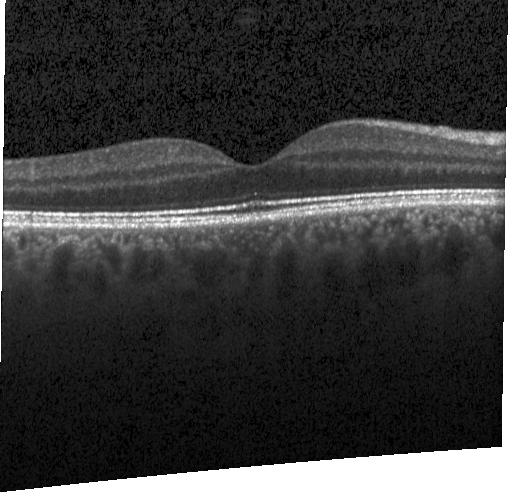
Optical coherence tomography B-scan
Impression: neither choroidal neovascularization, diabetic macular edema, nor drusen.